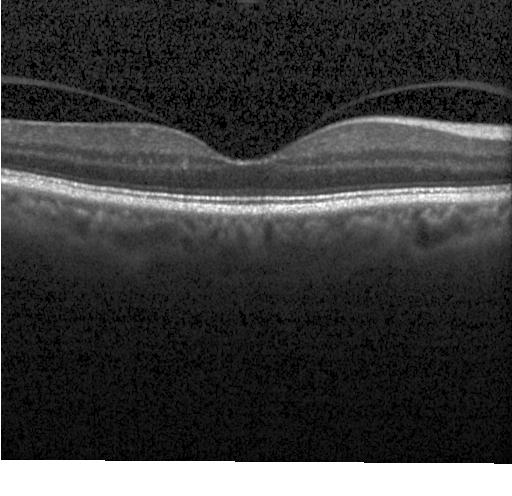 Through the macula · OCT line scan
Diagnosis: neither CNV, DME, nor drusen.